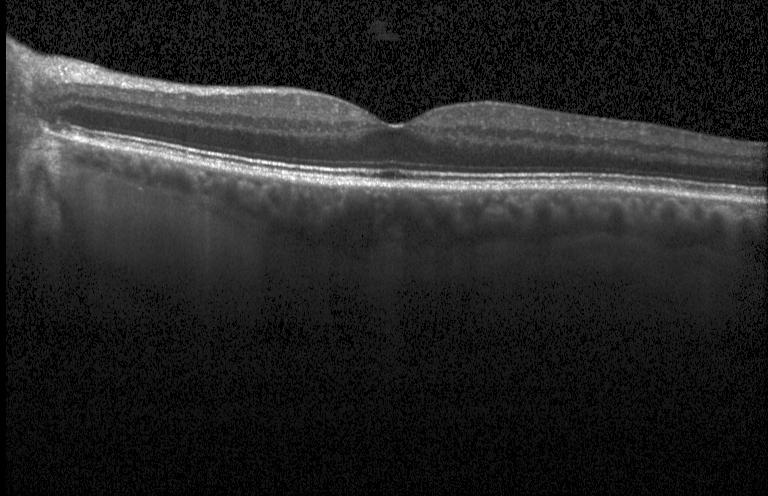 SD-OCT · through the macula · OCT line scan · instrument: Heidelberg Spectralis — Finding: no choroidal neovascularization, no diabetic macular edema, and no drusen.